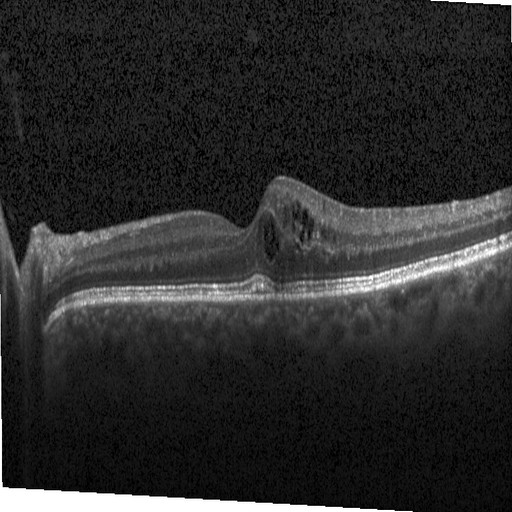
OCT line scan
This B-scan demonstrates DME.